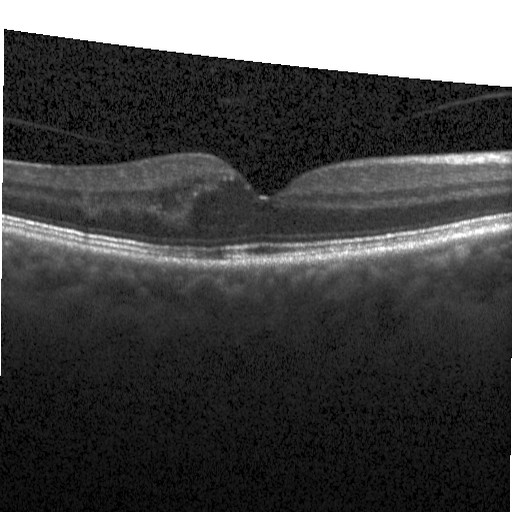
OCT line scan · spectral-domain OCT. Impression: diabetic macular edema (DME).